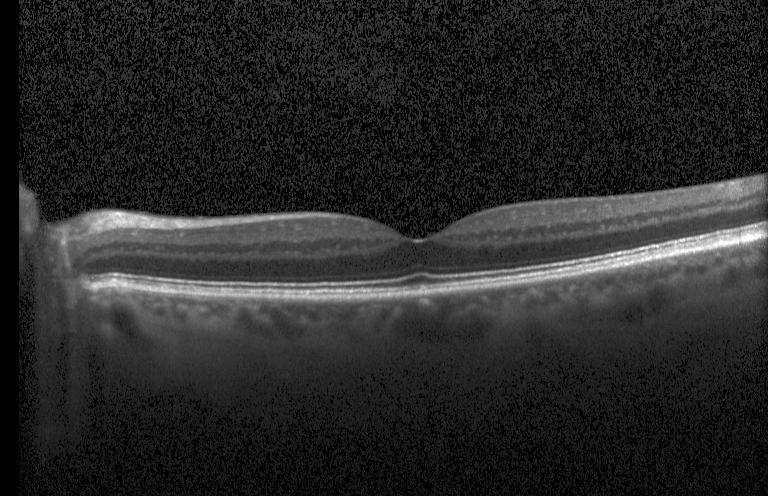
Centered on the fovea, instrument: Heidelberg Spectralis, OCT line scan — The scan shows no evidence of choroidal neovascularization, diabetic macular edema, or drusen.